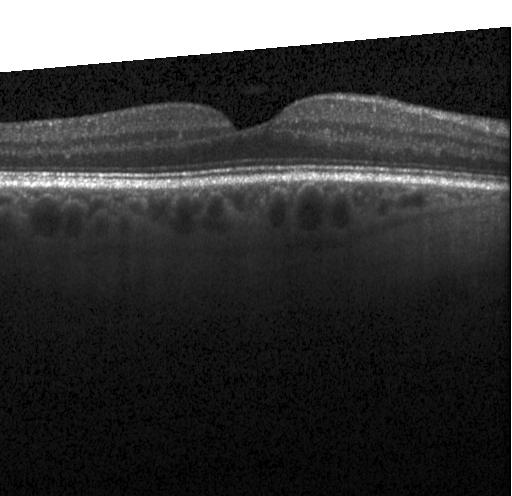

Retinal OCT B-scan — No choroidal neovascularization, diabetic macular edema, or drusen.